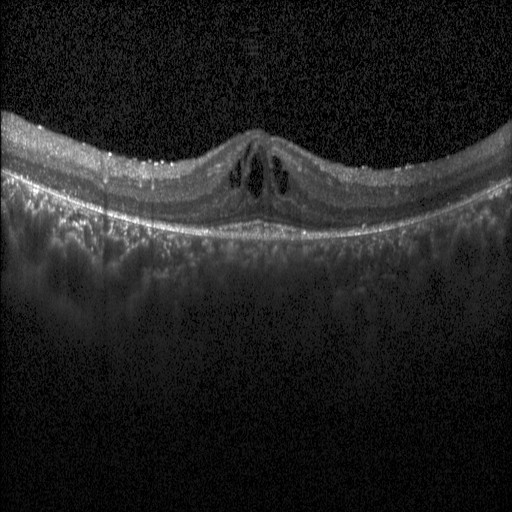 Diagnosis: diabetic macular edema (DME).